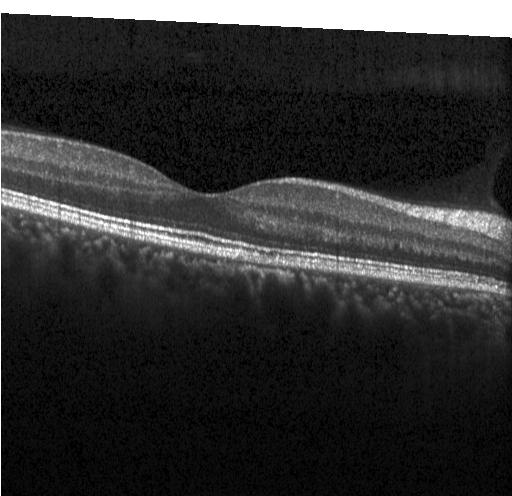
OCT B-scan. Acquired on a Heidelberg Spectralis. Centered on the fovea — Impression: no evidence of choroidal neovascularization, diabetic macular edema, or drusen.